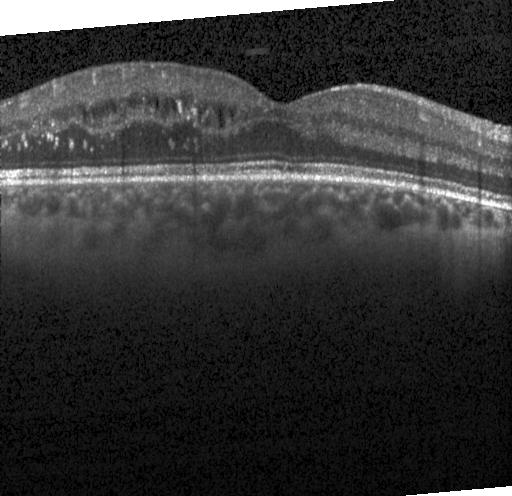 Impression: diabetic macular edema (DME).